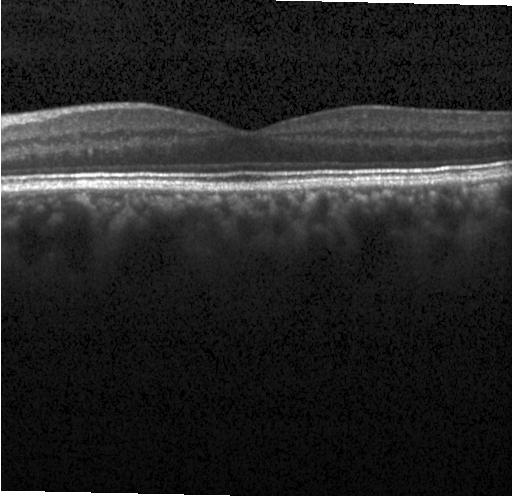
Optical coherence tomography scan. Impression: no evidence of CNV, DME, or drusen.